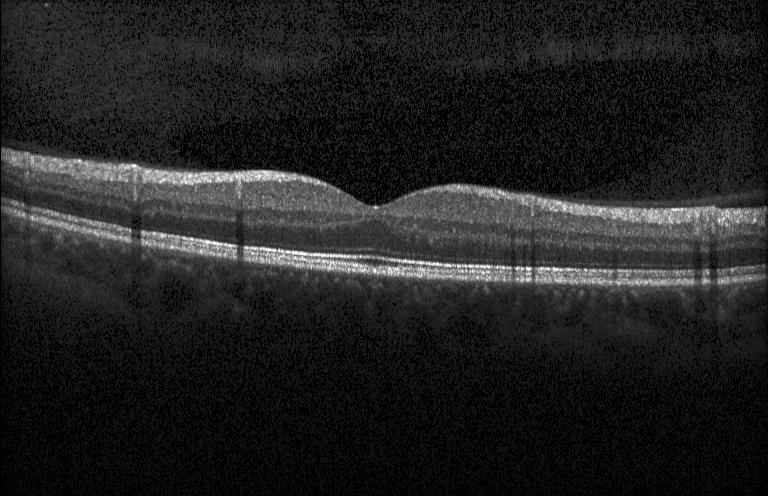
Optical coherence tomography B-scan, spectral-domain OCT, Heidelberg Spectralis OCT system, through the macula — The scan shows no CNV, no DME, and no drusen.